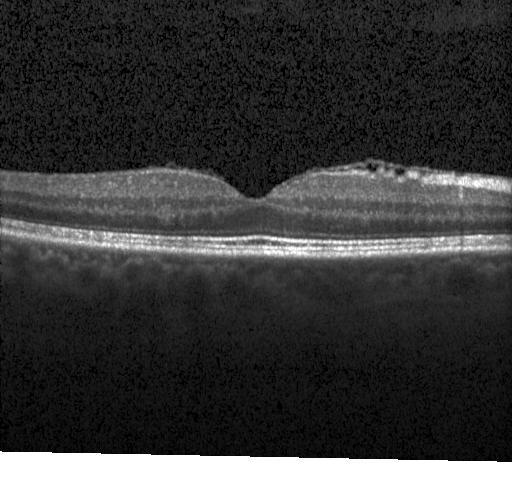
Diagnosis: neither CNV, DME, nor drusen.